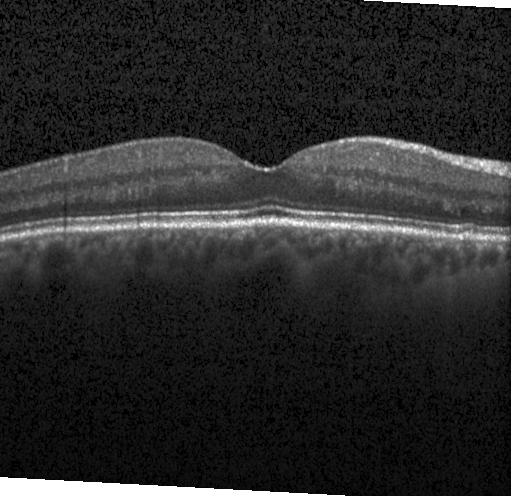 SD-OCT, retinal OCT B-scan, Heidelberg Spectralis OCT system. The scan shows neither choroidal neovascularization, diabetic macular edema, nor drusen.